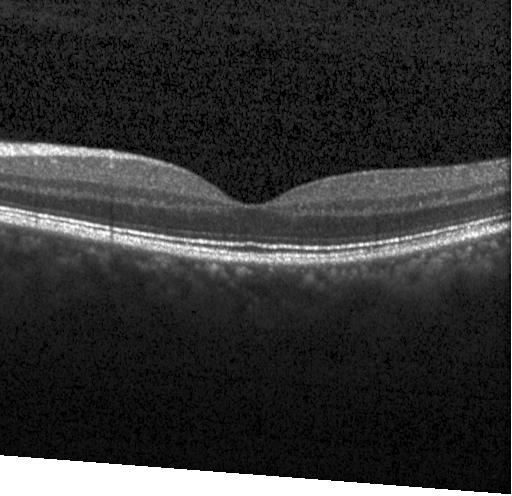

OCT B-scan. No choroidal neovascularization, diabetic macular edema, or drusen.